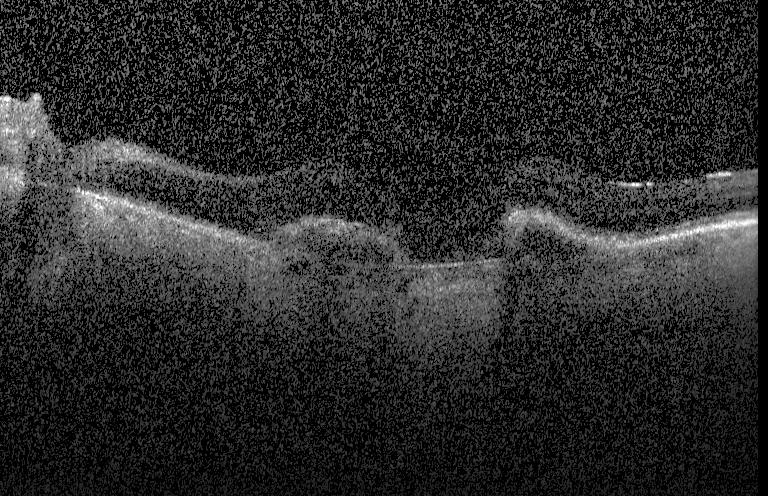 OCT B-scan, centered on the fovea, Heidelberg Spectralis, SD-OCT. This B-scan demonstrates choroidal neovascularization.